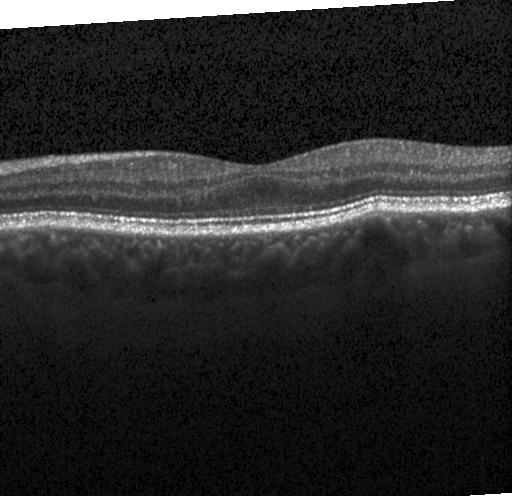

This B-scan demonstrates no evidence of choroidal neovascularization, diabetic macular edema, or drusen.